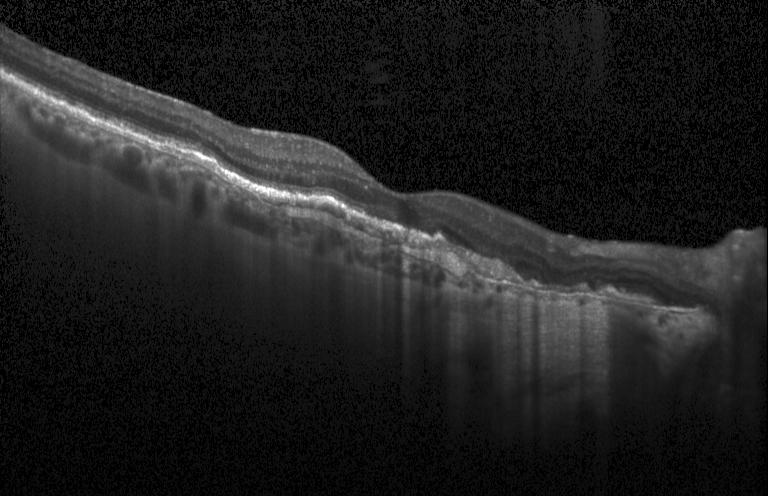
OCT scan showing a choroidal neovascular membrane.